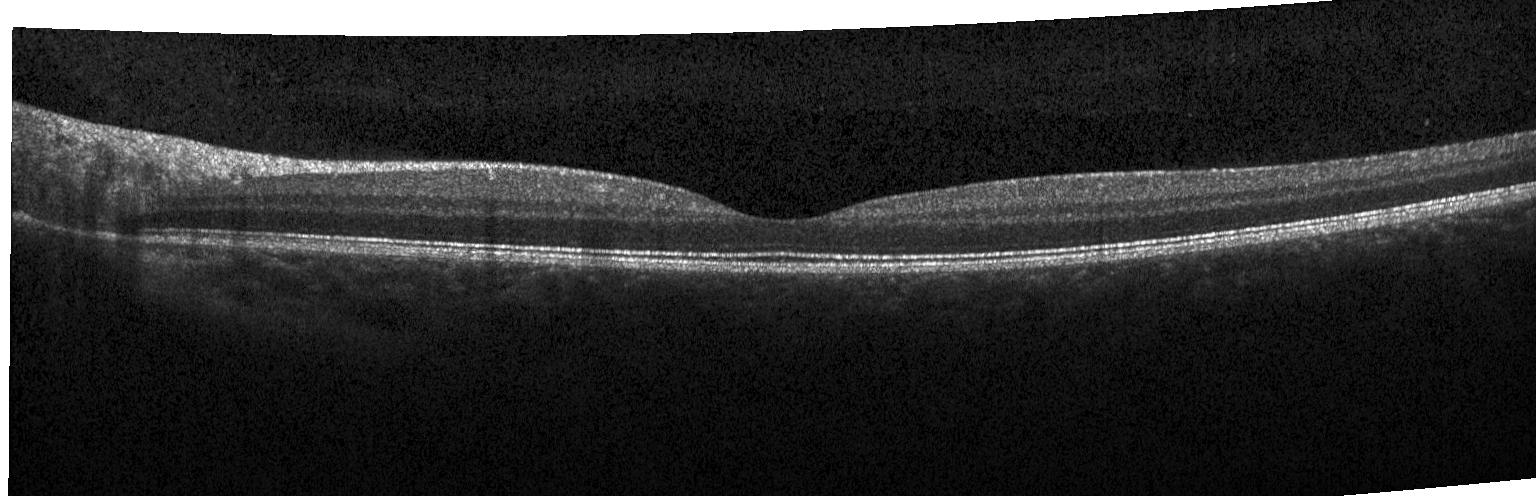

OCT B-scan · acquired on a Heidelberg Spectralis · fovea-centered
OCT finding: neither choroidal neovascularization, diabetic macular edema, nor drusen.